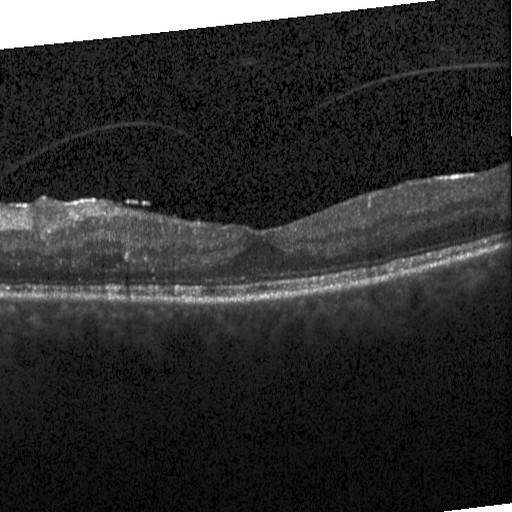
Retinal OCT B-scan · fovea-centered
This B-scan demonstrates DME.